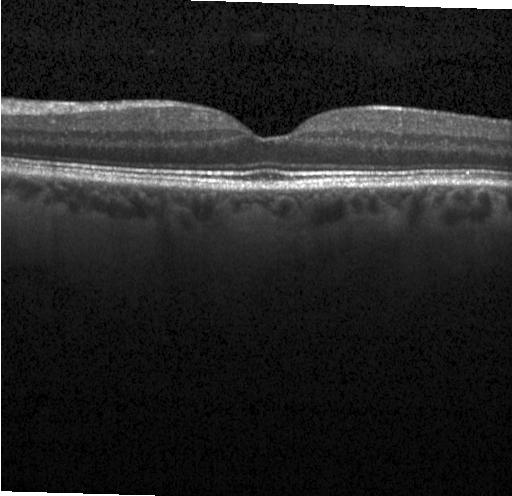
Fovea-centered; Heidelberg Spectralis; optical coherence tomography scan.
Impression: no choroidal neovascularization, no diabetic macular edema, and no drusen.